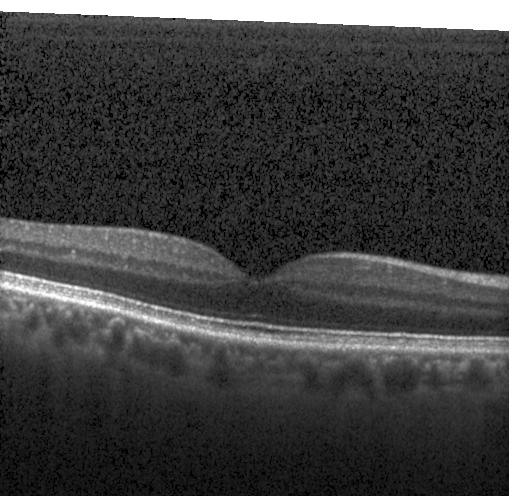 Optical coherence tomography scan · spectral-domain OCT
Macular OCT: no evidence of CNV, DME, or drusen.